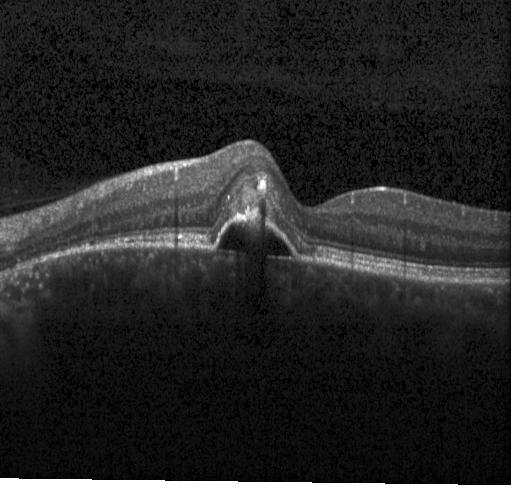

Retinal OCT cross-section — Impression: choroidal neovascularization.